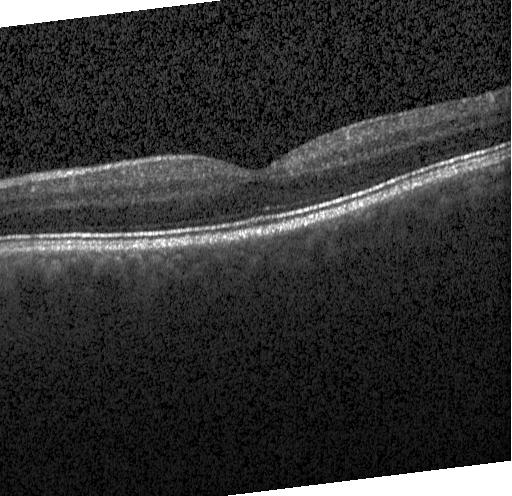

Diagnosis: neither choroidal neovascularization, diabetic macular edema, nor drusen.